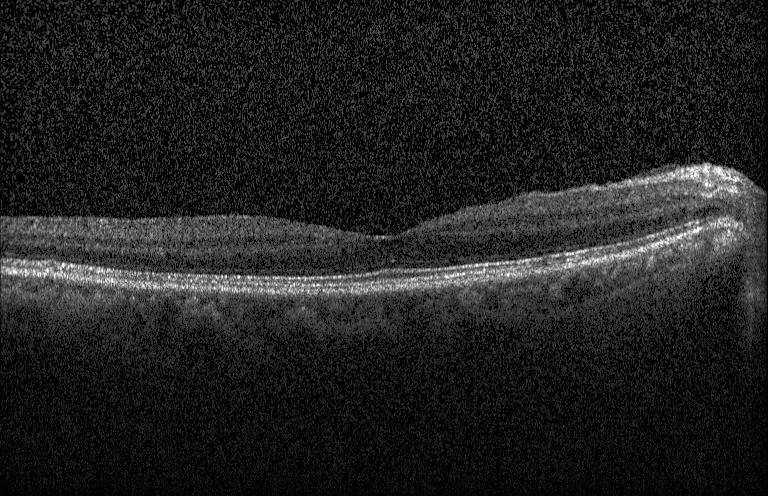

Optical coherence tomography scan. Fovea-centered.
Impression: neither choroidal neovascularization, diabetic macular edema, nor drusen.